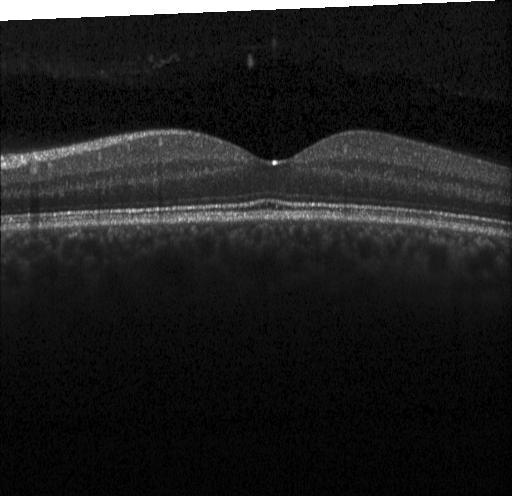 OCT line scan — Diagnosis: no choroidal neovascularization, no diabetic macular edema, and no drusen.